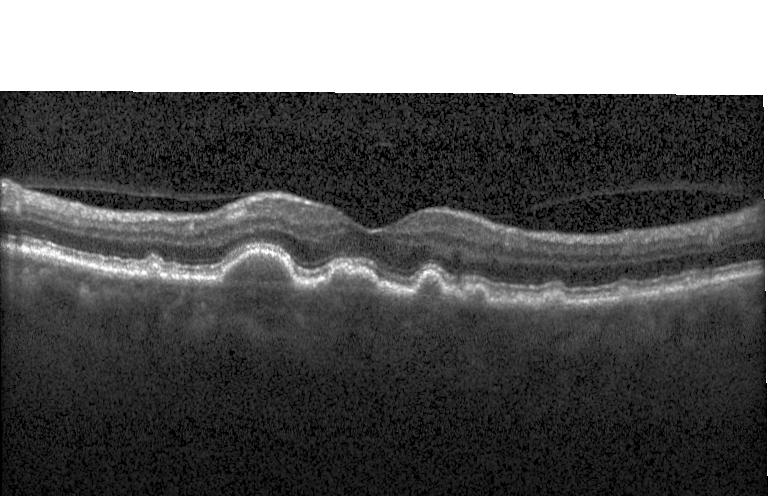
Through the macula; OCT line scan; acquired on a Heidelberg Spectralis; SD-OCT. Drusen.